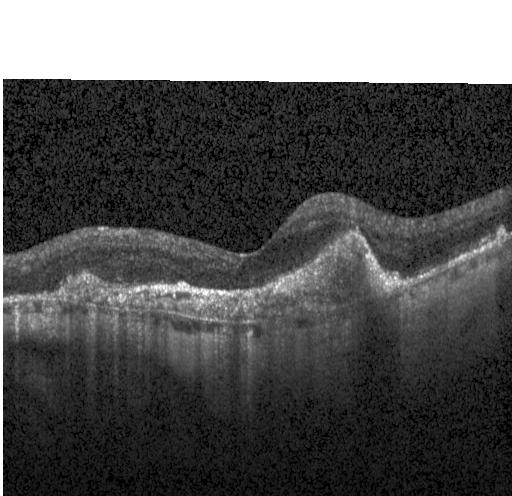
Macular OCT: a choroidal neovascular membrane.